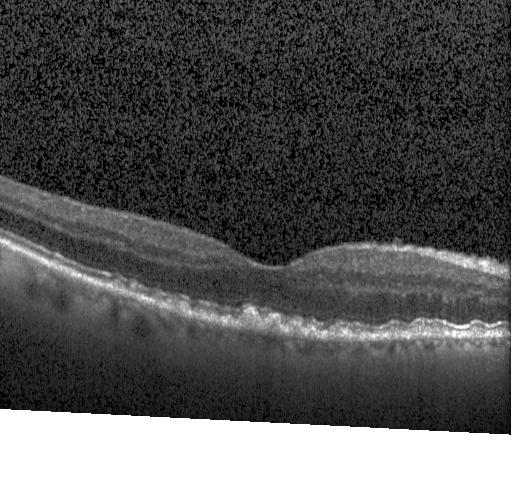
Instrument: Heidelberg Spectralis. OCT B-scan. Spectral-domain OCT — Finding: drusen.